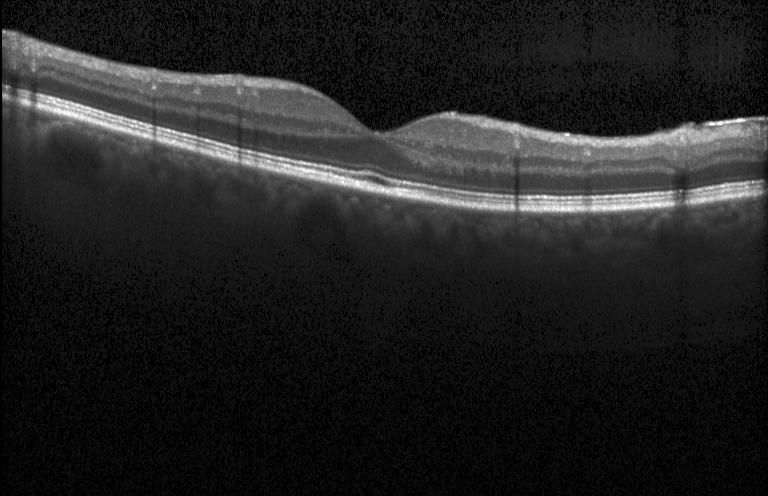
Diagnosis: no evidence of choroidal neovascularization, diabetic macular edema, or drusen.